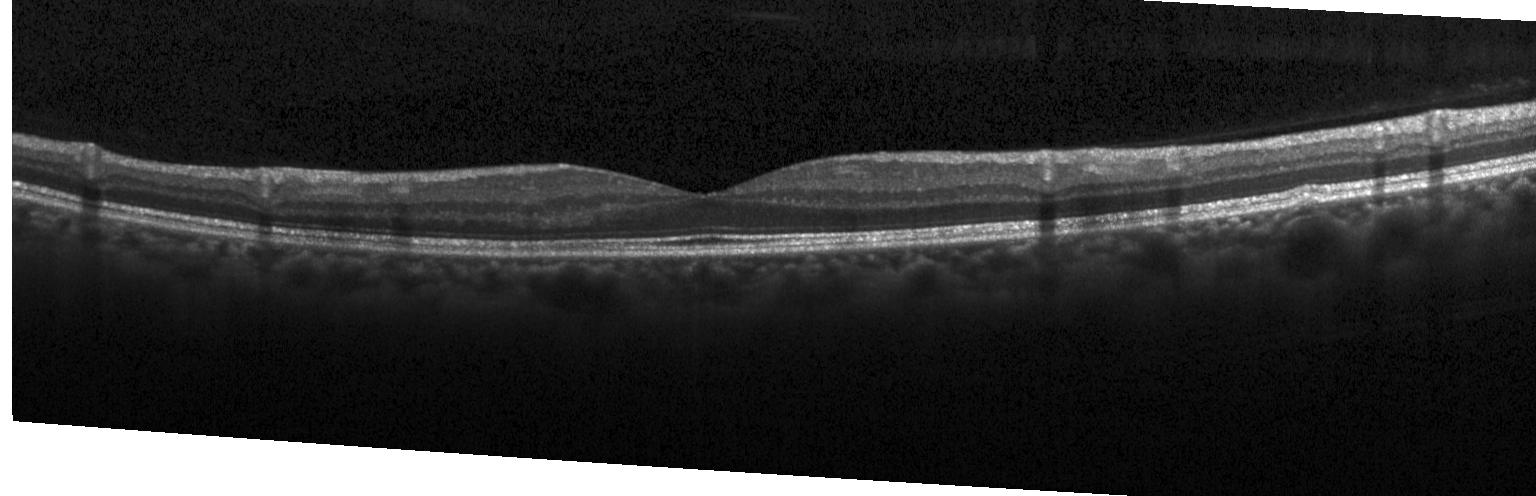

Spectral-domain optical coherence tomography; Heidelberg Spectralis OCT system; macular scan; optical coherence tomography scan
Impression: no evidence of choroidal neovascularization, diabetic macular edema, or drusen.